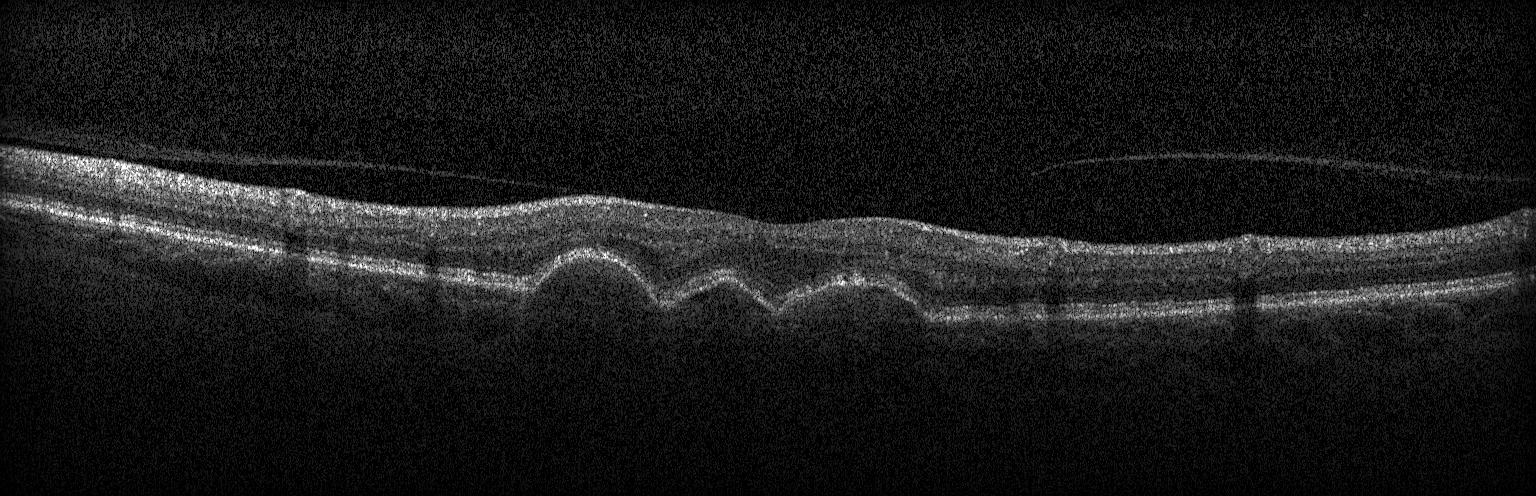

Fovea-centered; spectral-domain optical coherence tomography; retinal OCT B-scan; Heidelberg Spectralis OCT system.
Diagnosis: a choroidal neovascular membrane.